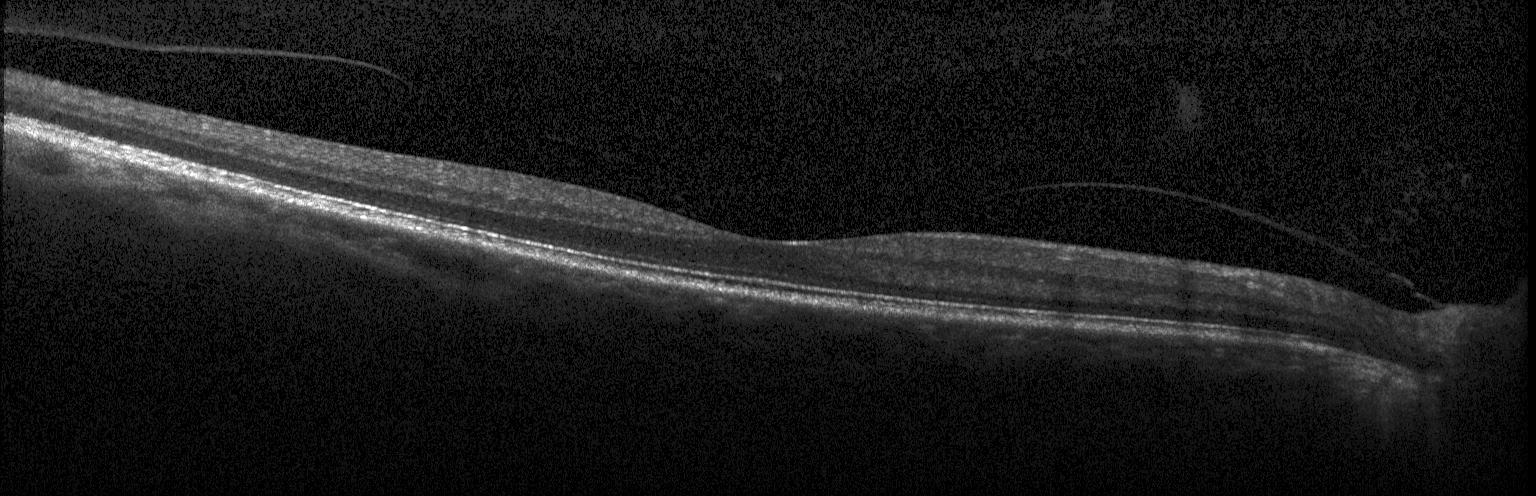

OCT B-scan showing no CNV, DME, or drusen.